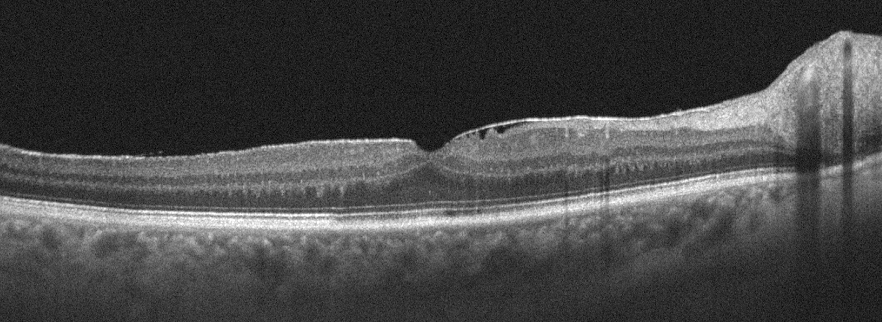
Right eye, retinal OCT B-scan, acquired on an Optovue Avanti RTVue XR — Finding: epiretinal membrane.